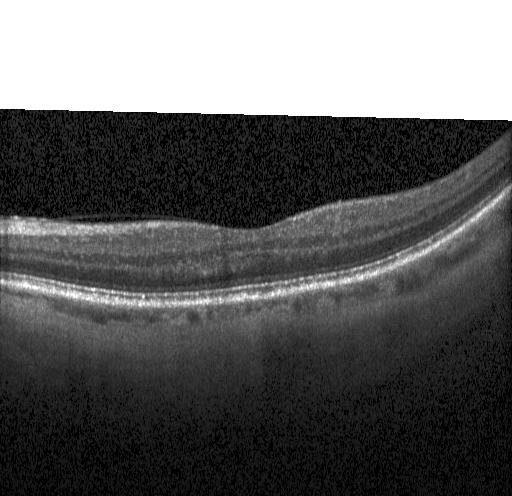
Retinal OCT cross-section. SD-OCT
Finding: no evidence of CNV, DME, or drusen.